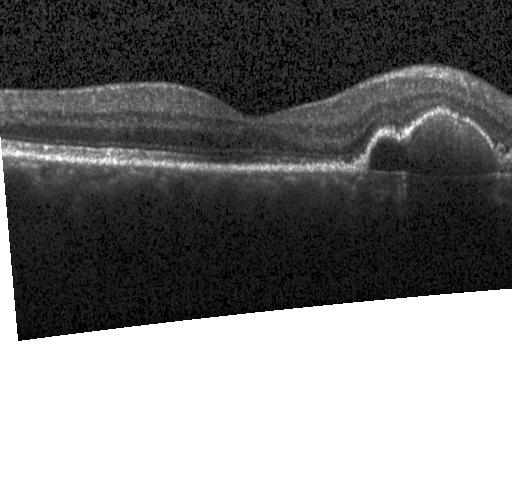 OCT scan showing CNV.